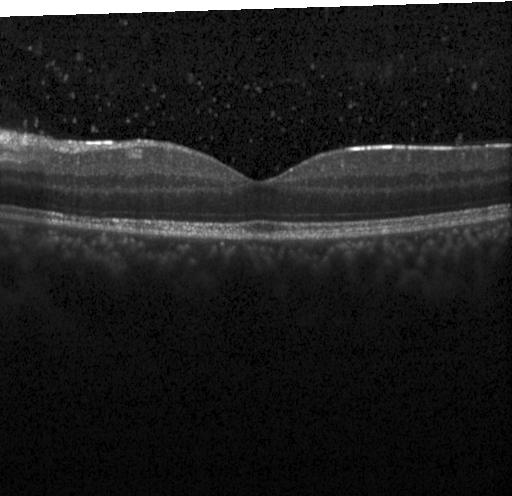
Impression: neither CNV, DME, nor drusen.